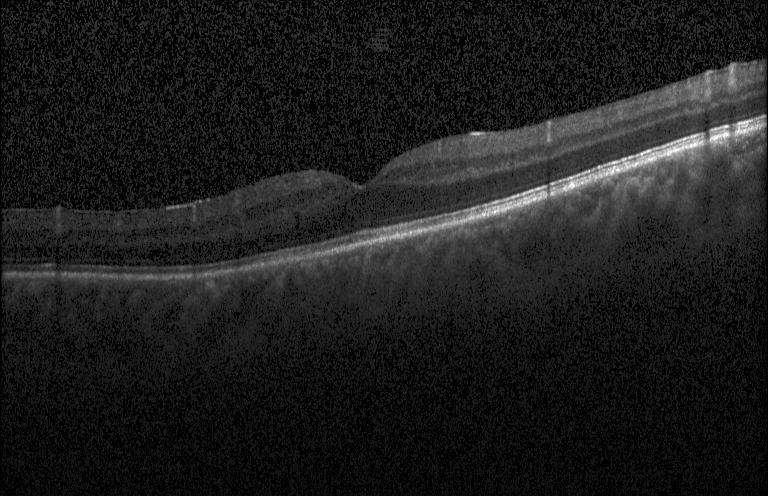 Optical coherence tomography B-scan — Impression: no CNV, DME, or drusen.